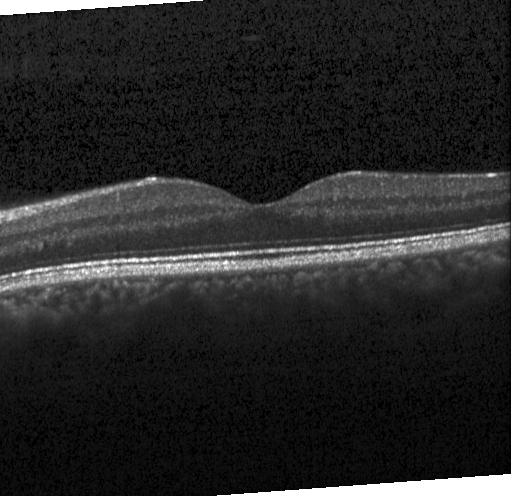

OCT finding: no choroidal neovascularization, no diabetic macular edema, and no drusen.